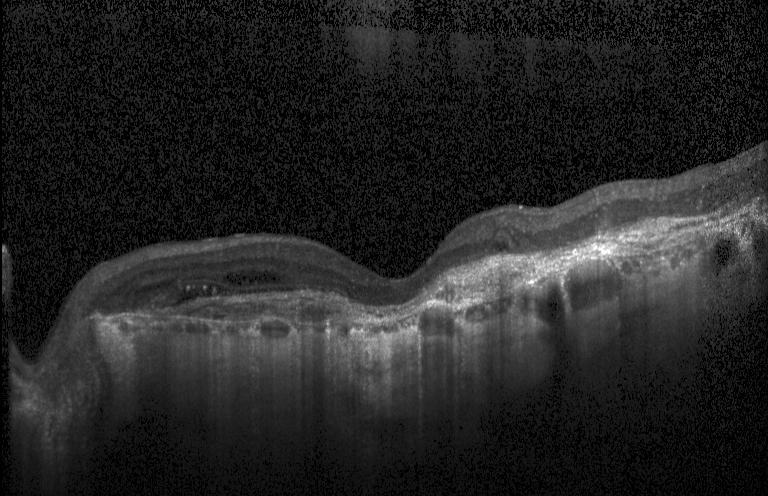
OCT scan showing a choroidal neovascular membrane.